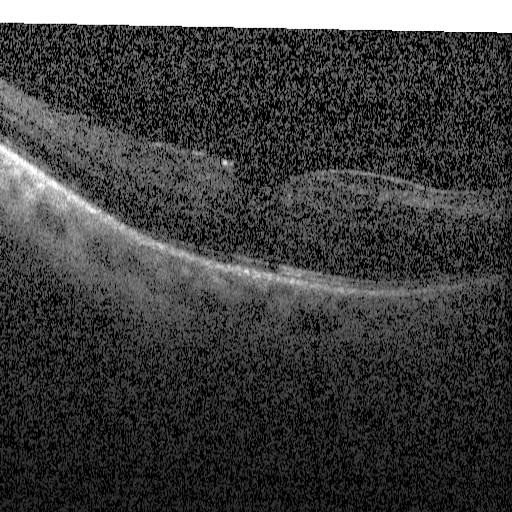 Spectral-domain OCT B-scan: diabetic macular edema.